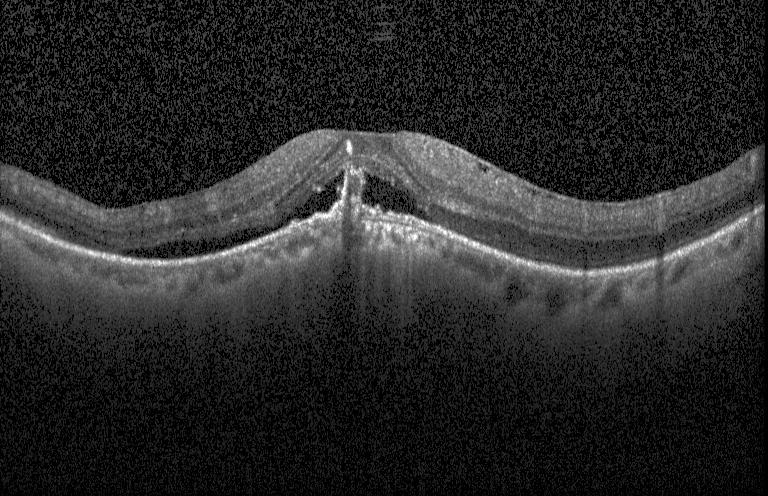
Retinal OCT B-scan. Heidelberg Spectralis.
Impression: a choroidal neovascular membrane.